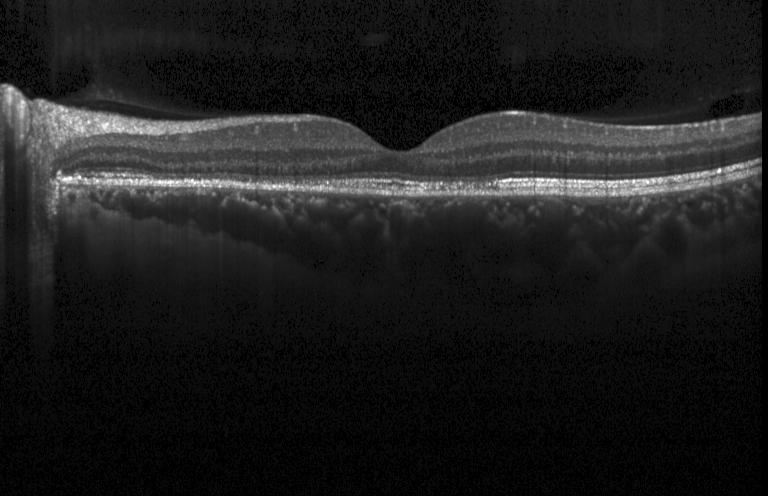

Assessment: no choroidal neovascularization, no diabetic macular edema, and no drusen.